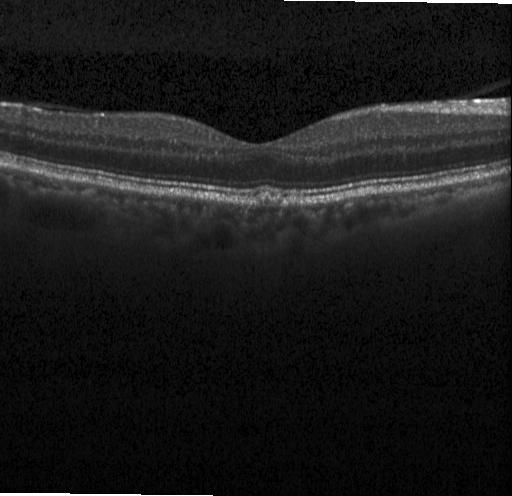 Diagnosis: drusen.